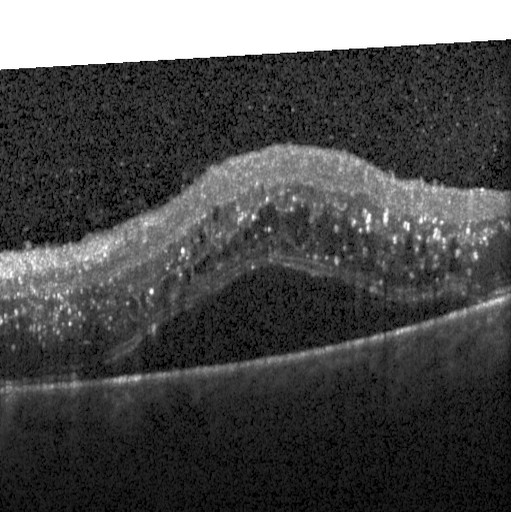 Spectral-domain OCT B-scan: DME.